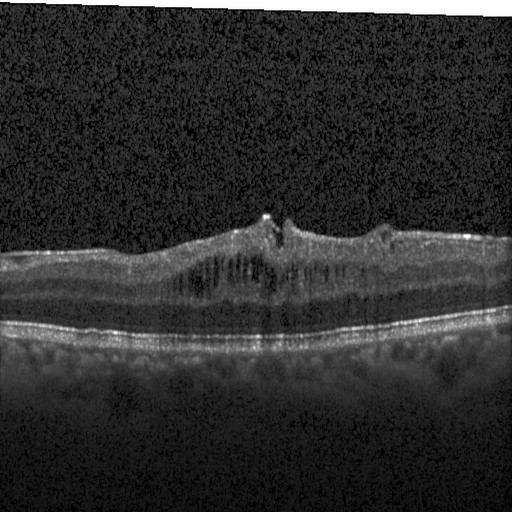

Through the macula, optical coherence tomography B-scan, acquired on a Heidelberg Spectralis. DME.